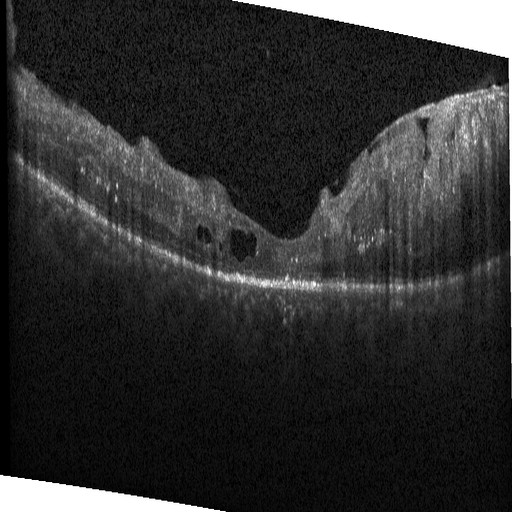

Heidelberg Spectralis; OCT B-scan — Macular OCT: DME.